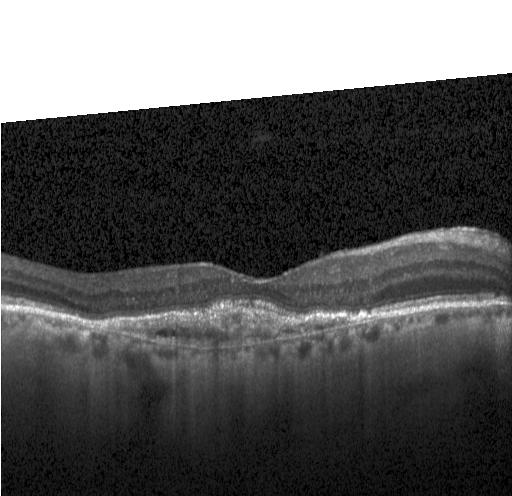

OCT B-scan. Horizontal scan through the fovea. Instrument: Heidelberg Spectralis. Spectral-domain optical coherence tomography
This B-scan demonstrates CNV.